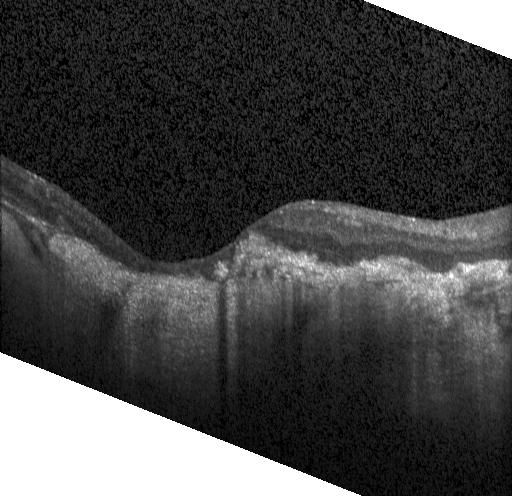
Macular OCT demonstrating choroidal neovascularization (CNV).